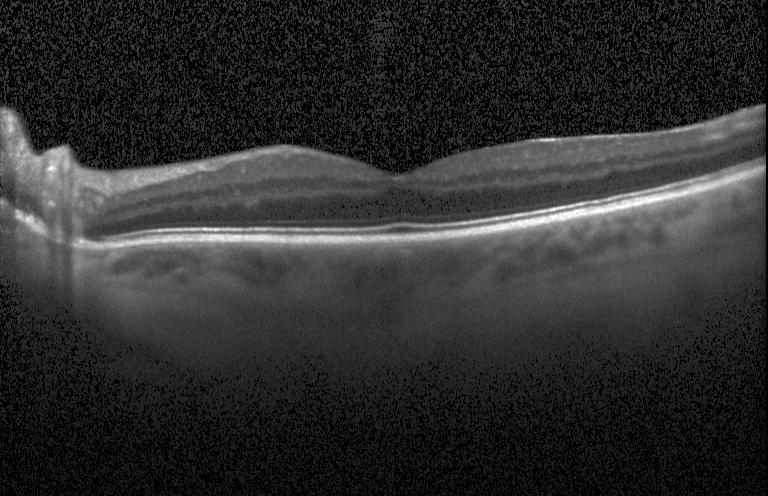
Centered on the fovea; spectral-domain optical coherence tomography; retinal OCT cross-section; Heidelberg Spectralis — Dx: neither CNV, DME, nor drusen.